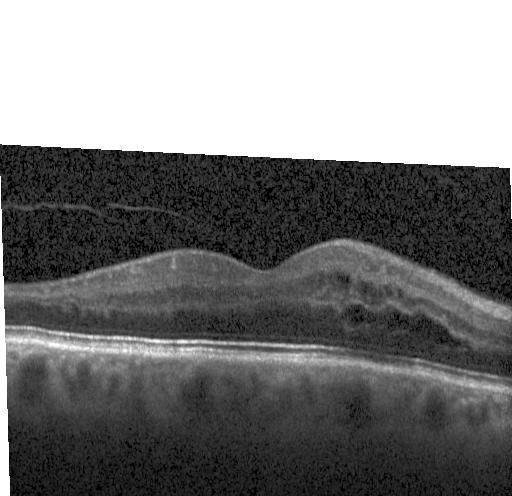

OCT finding: DME.